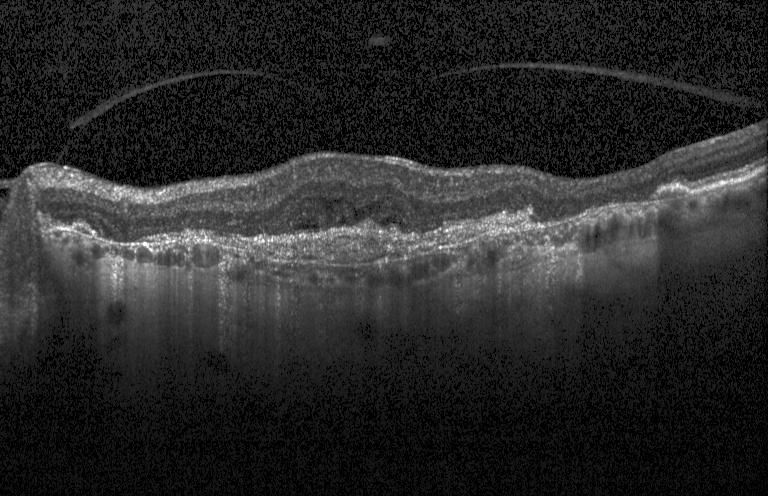 Spectral-domain OCT. Optical coherence tomography scan. Horizontal scan through the fovea. Heidelberg Spectralis OCT system. Finding: a choroidal neovascular membrane.